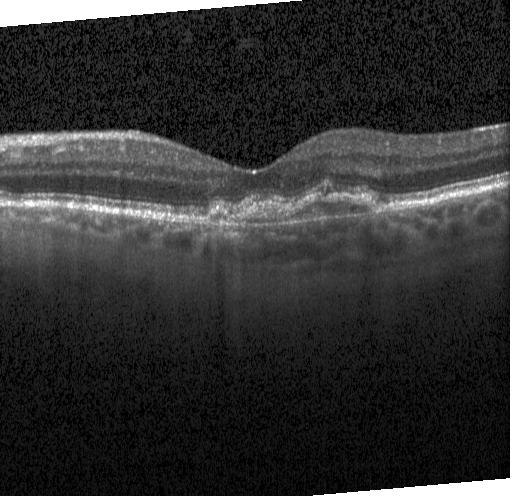 SD-OCT, optical coherence tomography scan, centered on the fovea — Impression: choroidal neovascularization (CNV).